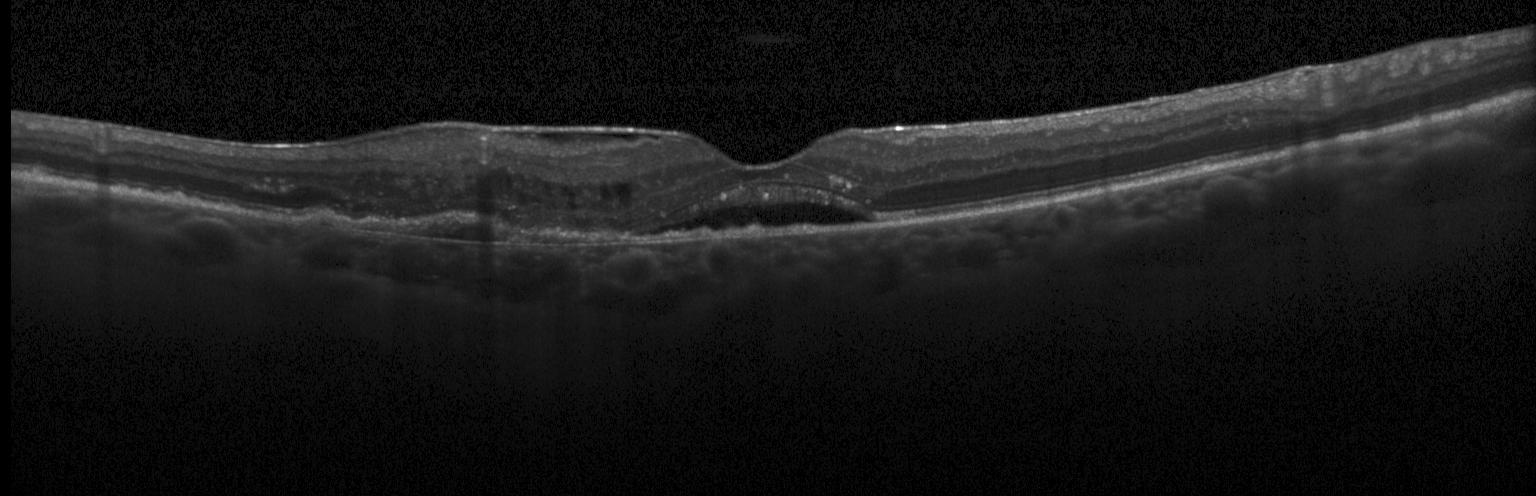 Impression: a choroidal neovascular membrane.